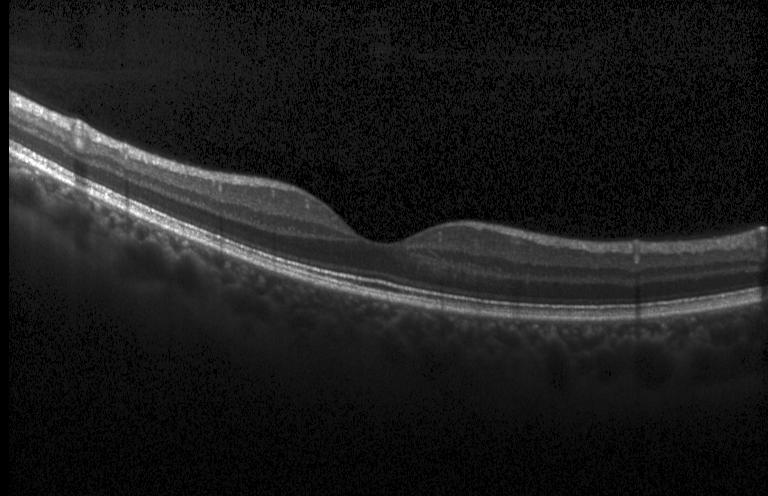
OCT B-scan showing no evidence of choroidal neovascularization, diabetic macular edema, or drusen.